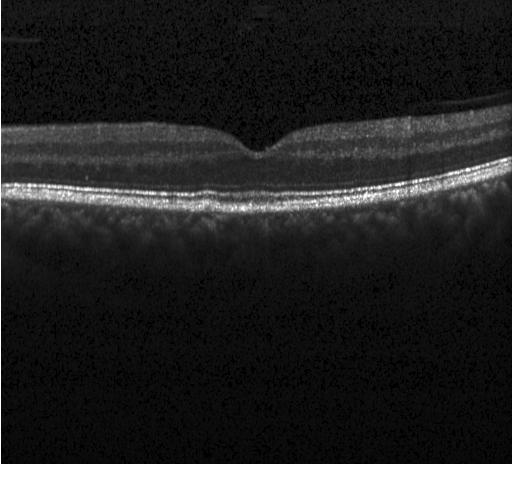

Spectral-domain OCT B-scan: multiple drusen.